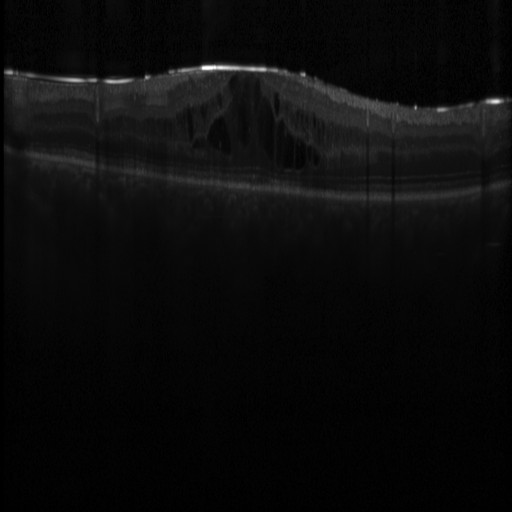

OCT B-scan; spectral-domain OCT; horizontal scan through the fovea; instrument: Heidelberg Spectralis — Diagnosis: diabetic macular edema.